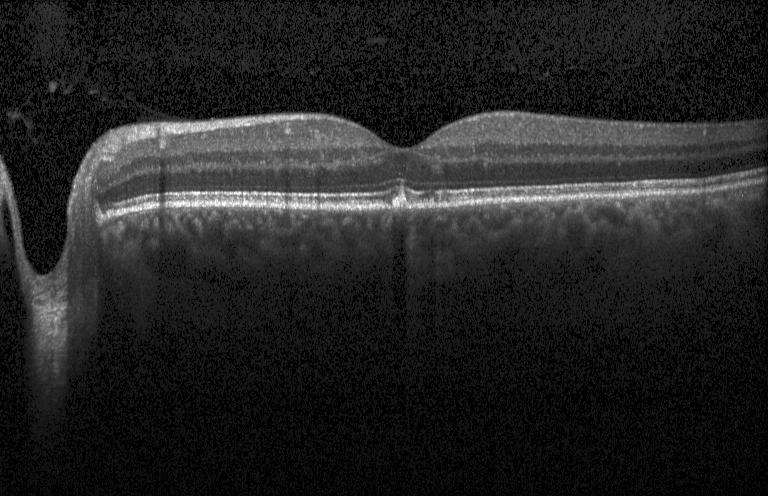
Spectral-domain optical coherence tomography. OCT line scan — This B-scan demonstrates sub-RPE drusenoid deposits.